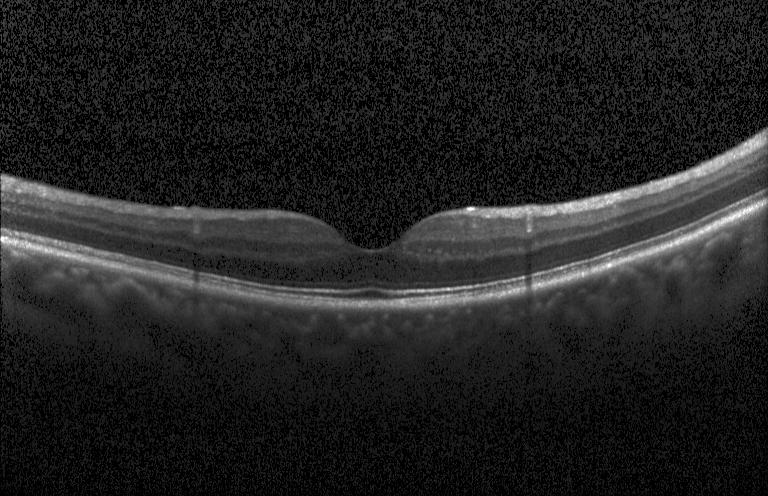 Heidelberg Spectralis. Macular scan. Optical coherence tomography B-scan. Impression: no evidence of choroidal neovascularization, diabetic macular edema, or drusen.